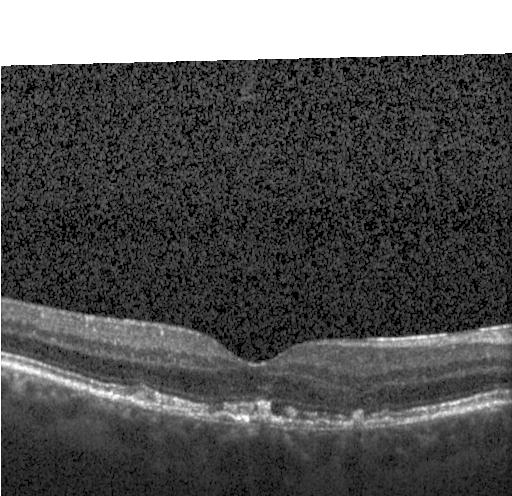

Diagnosis: a choroidal neovascular membrane.